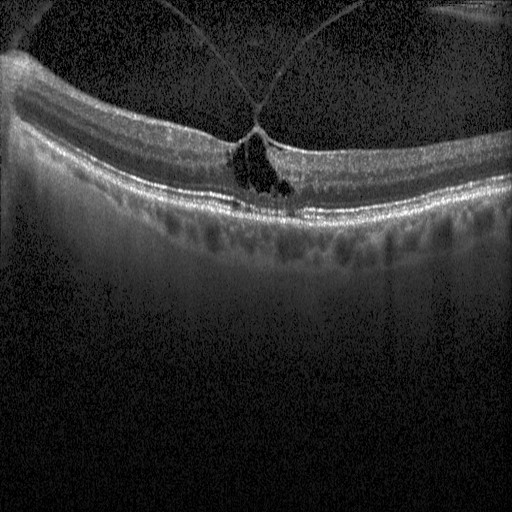 Through the macula. SD-OCT. Retinal OCT B-scan. Impression: diabetic macular edema.